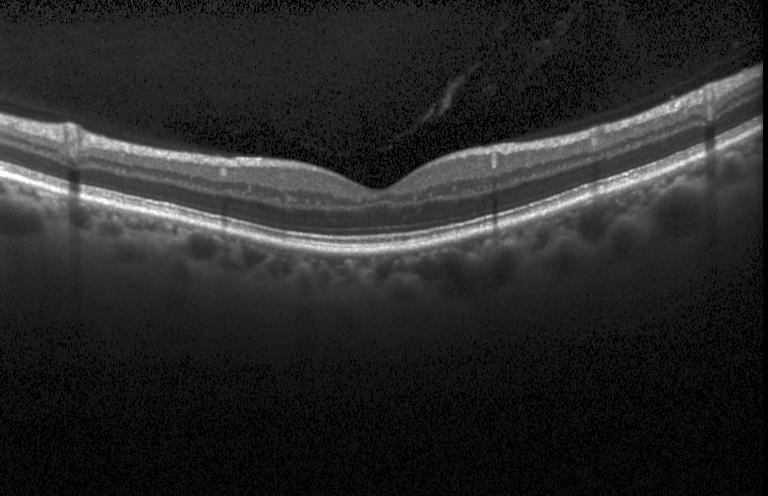
Dx: no evidence of choroidal neovascularization, diabetic macular edema, or drusen.